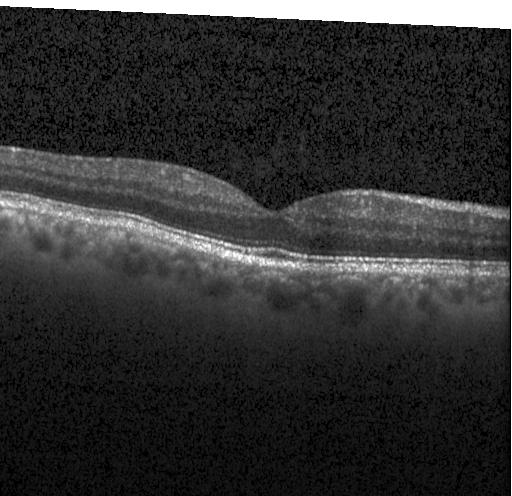 Finding: no evidence of choroidal neovascularization, diabetic macular edema, or drusen.